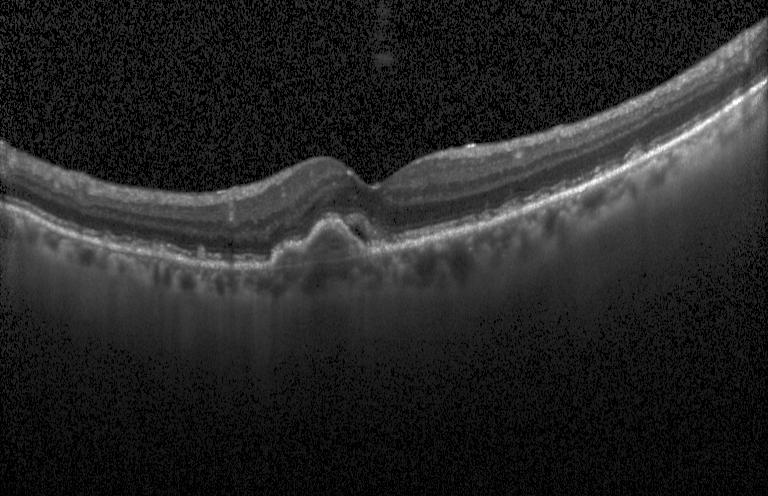
Spectral-domain OCT; retinal OCT cross-section; centered on the fovea; instrument: Heidelberg Spectralis
Impression: a choroidal neovascular membrane.